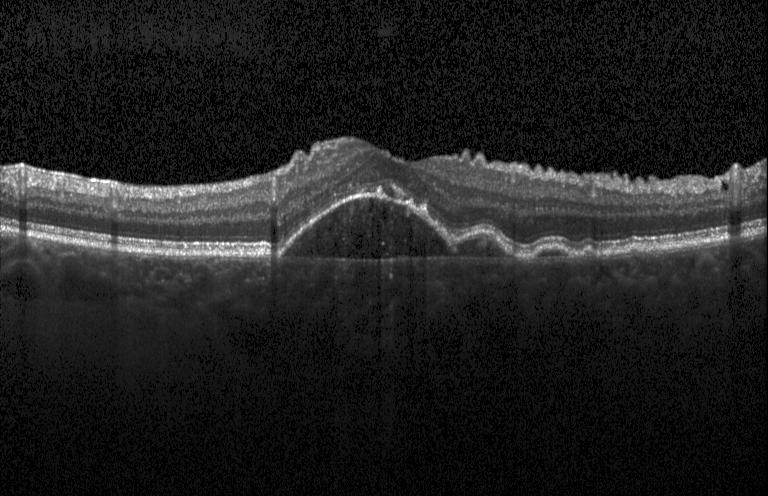
Assessment: a choroidal neovascular membrane.